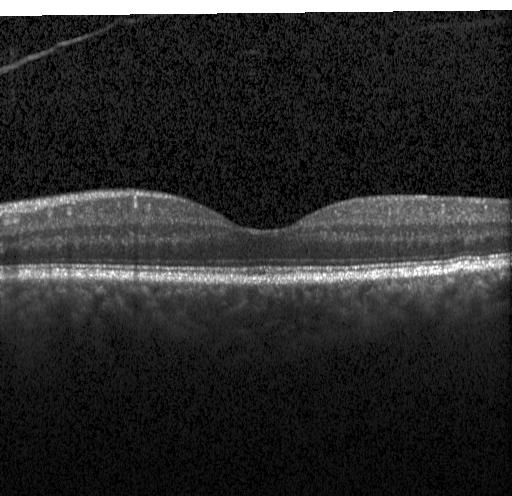 Spectral-domain OCT B-scan: no choroidal neovascularization, diabetic macular edema, or drusen.